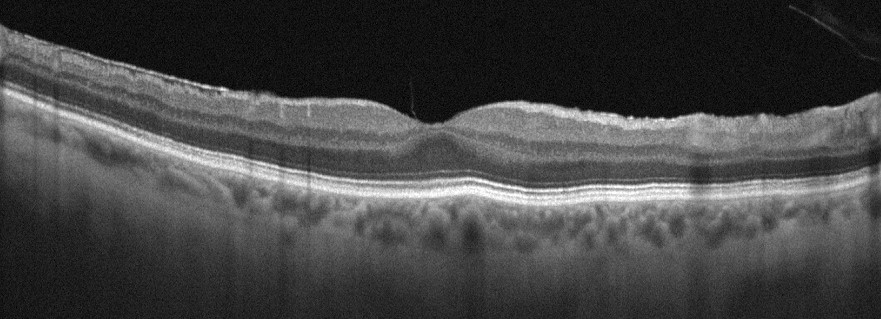 OCT line scan — Diagnosis: ERM.